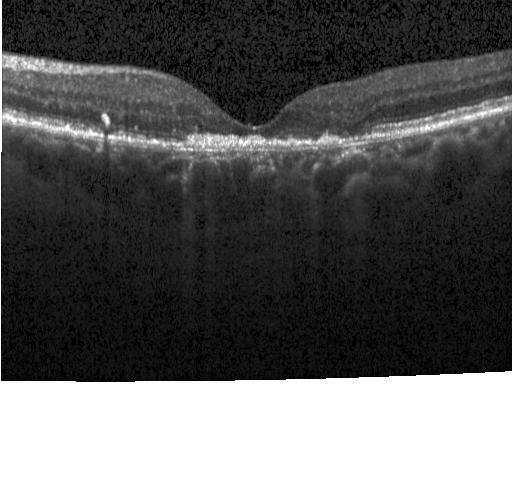 OCT finding: choroidal neovascularization (CNV).